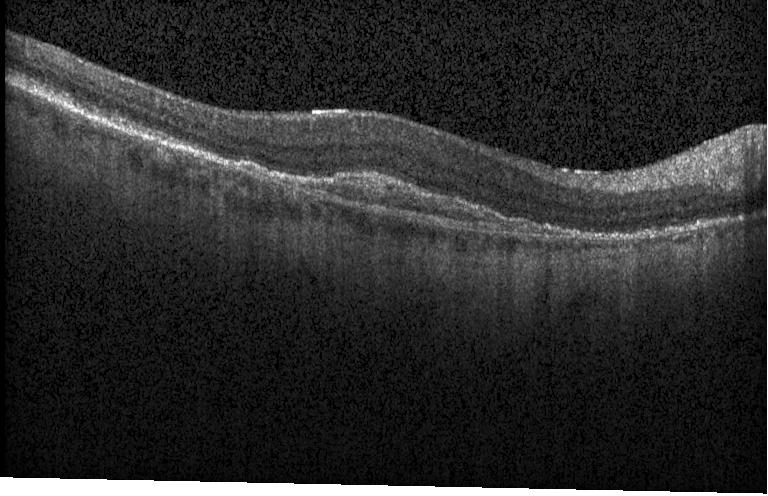
Optical coherence tomography scan; macular scan; Heidelberg Spectralis; spectral-domain optical coherence tomography
The scan shows a choroidal neovascular membrane.